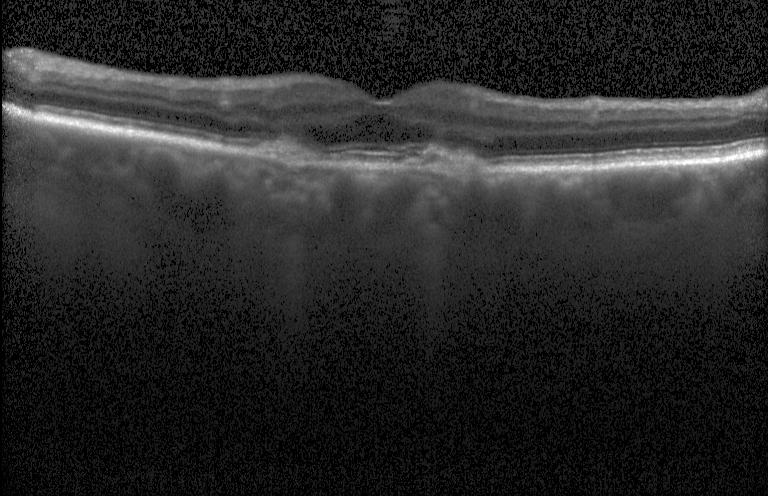

OCT finding: a choroidal neovascular membrane.